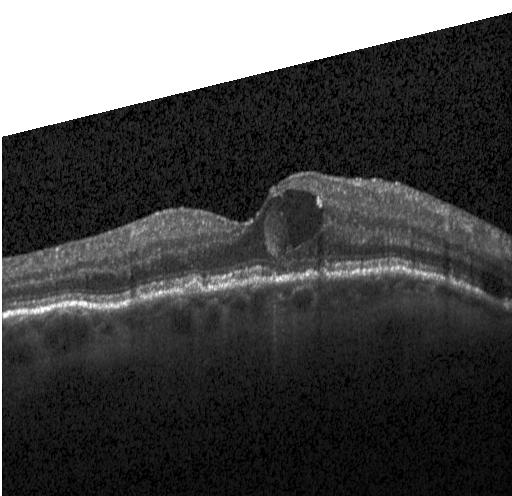

Through the macula. OCT line scan
Dx: a choroidal neovascular membrane.